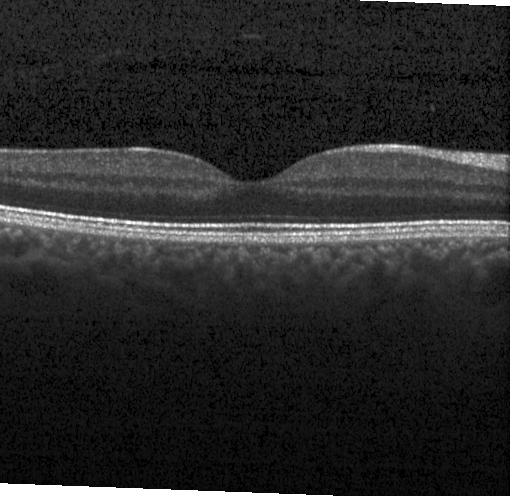 Optical coherence tomography scan. The scan shows no choroidal neovascularization, diabetic macular edema, or drusen.